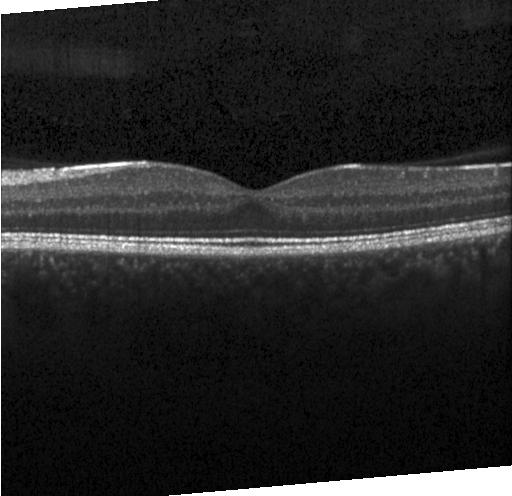

Retinal OCT cross-section showing neither choroidal neovascularization, diabetic macular edema, nor drusen.